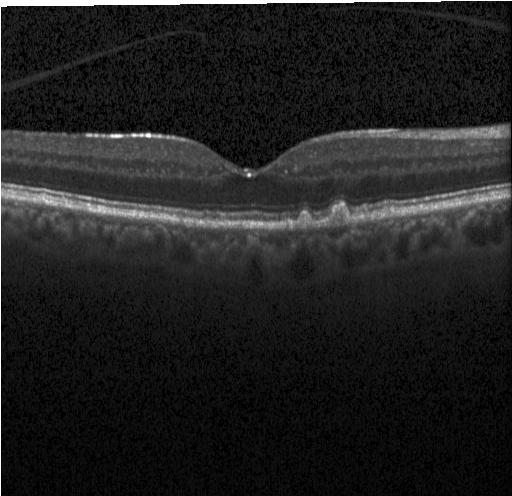
OCT B-scan showing sub-RPE drusenoid deposits.